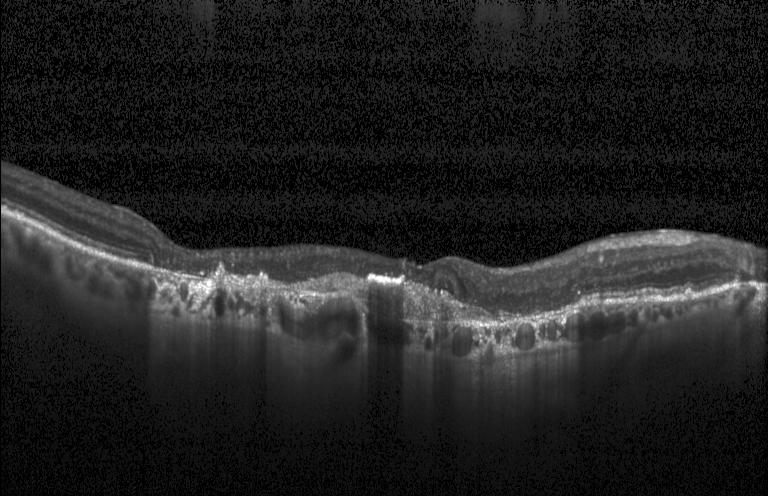

Optical coherence tomography B-scan, SD-OCT, Heidelberg Spectralis, macular scan. Impression: choroidal neovascularization (CNV).